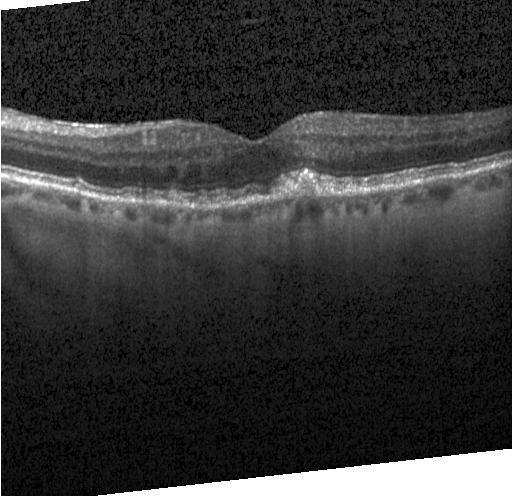

SD-OCT; centered on the fovea; retinal OCT cross-section.
Impression: drusen.